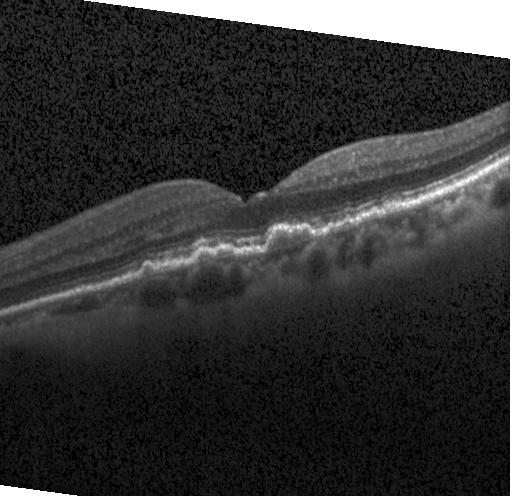

OCT line scan · instrument: Heidelberg Spectralis — Diagnosis: drusen.